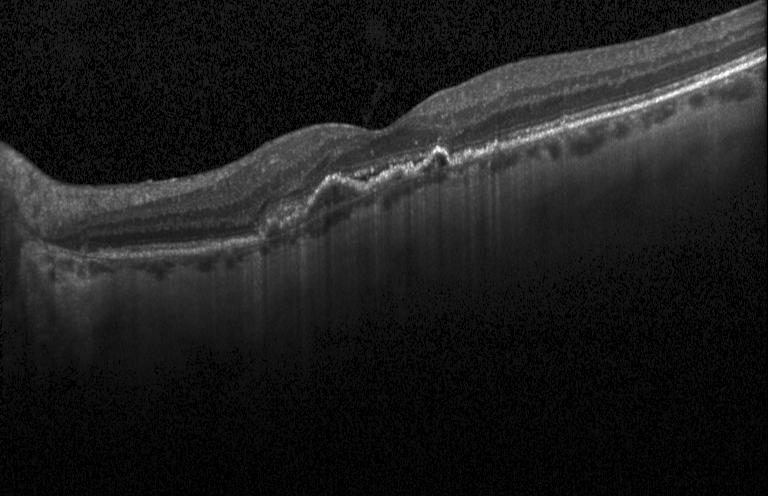

Finding: choroidal neovascularization (CNV).